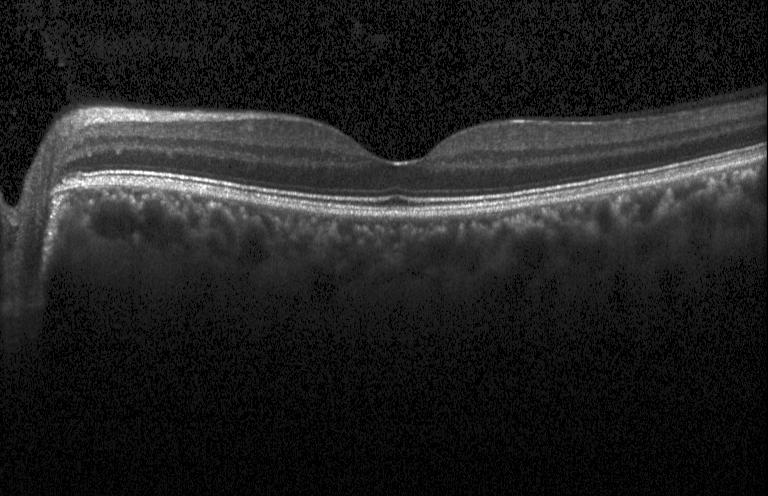
Finding: no evidence of choroidal neovascularization, diabetic macular edema, or drusen.